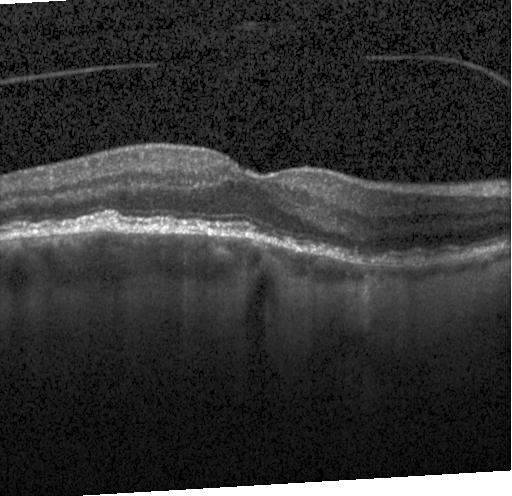
Retinal OCT cross-section; through the macula; Heidelberg Spectralis; spectral-domain optical coherence tomography.
The scan shows sub-RPE drusenoid deposits.